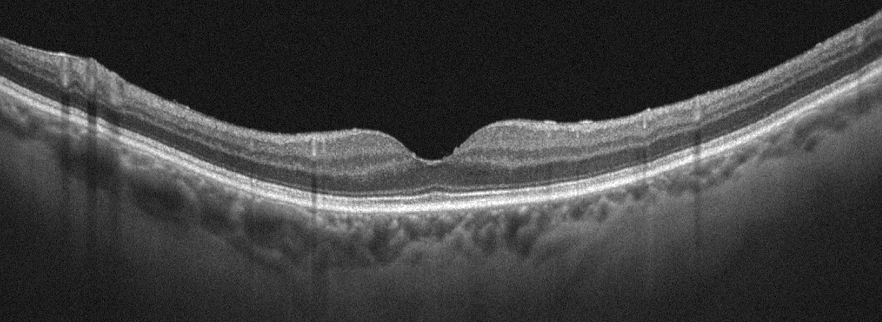 OCT line scan; right eye.
Macular OCT: absence of AMD, DME, ERM, RAO, RVO, and vitreomacular interface disease.